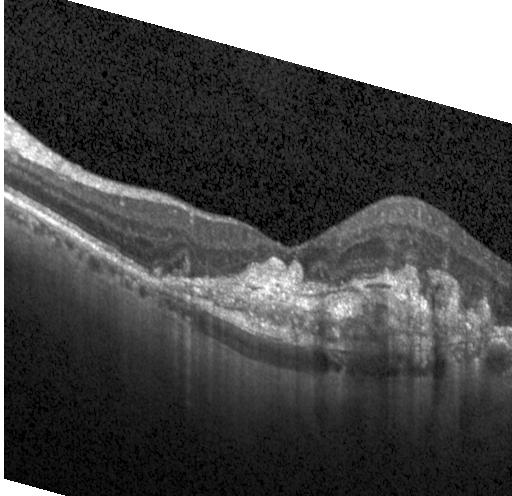 OCT scan showing a choroidal neovascular membrane.